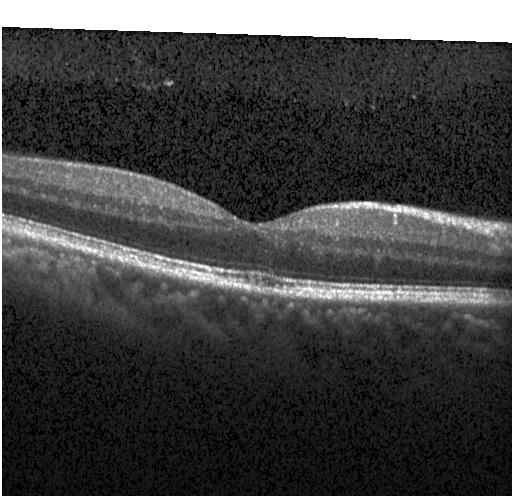 Macular scan; instrument: Heidelberg Spectralis; SD-OCT; OCT line scan. Finding: no choroidal neovascularization, diabetic macular edema, or drusen.